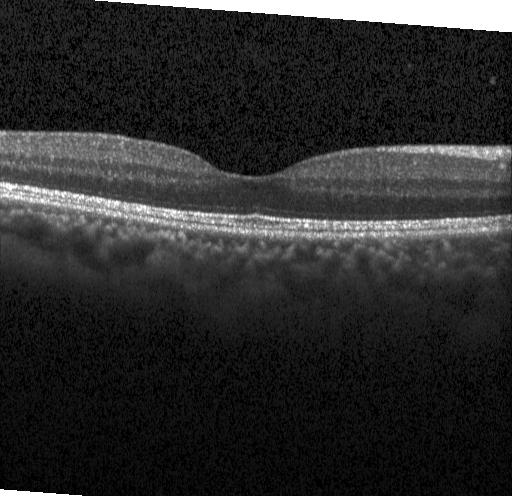

This B-scan demonstrates no CNV, no DME, and no drusen.